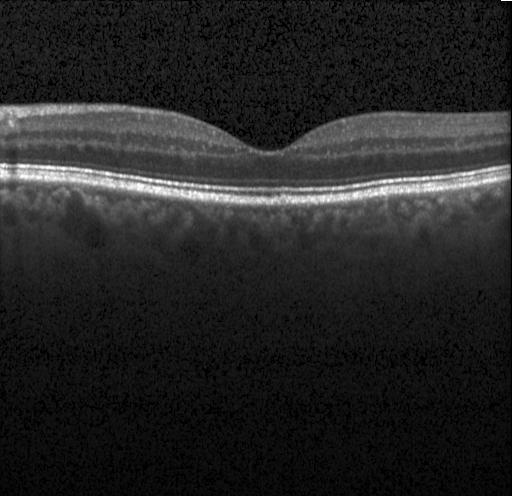

Horizontal scan through the fovea, OCT B-scan
This B-scan demonstrates no evidence of choroidal neovascularization, diabetic macular edema, or drusen.